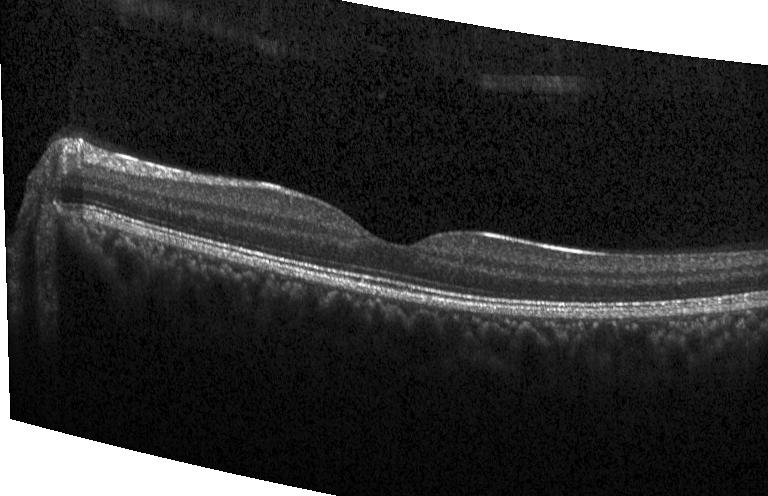

Optical coherence tomography B-scan; Heidelberg Spectralis OCT system. Finding: no evidence of choroidal neovascularization, diabetic macular edema, or drusen.